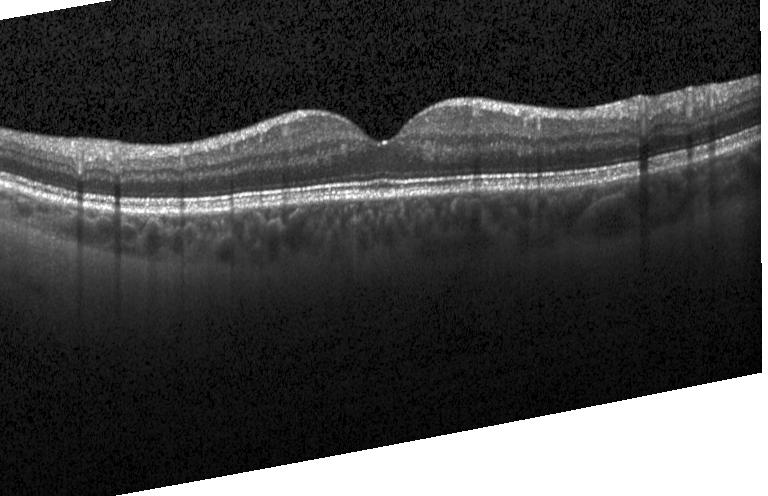

Optical coherence tomography scan — The scan shows no CNV, no DME, and no drusen.